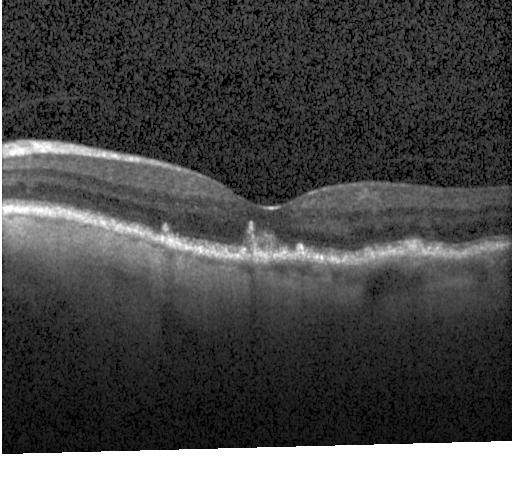

Spectral-domain optical coherence tomography. Heidelberg Spectralis. Retinal OCT cross-section.
Finding: sub-RPE drusenoid deposits.